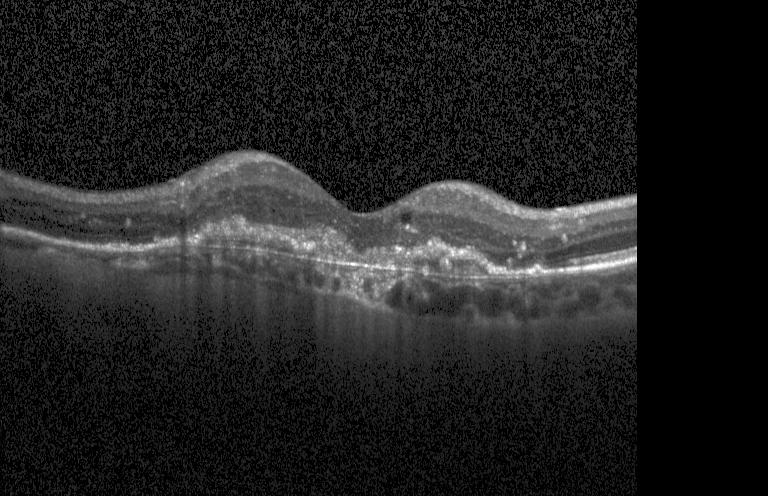
Macular scan, OCT B-scan, SD-OCT, acquired on a Heidelberg Spectralis.
Macular OCT: CNV.